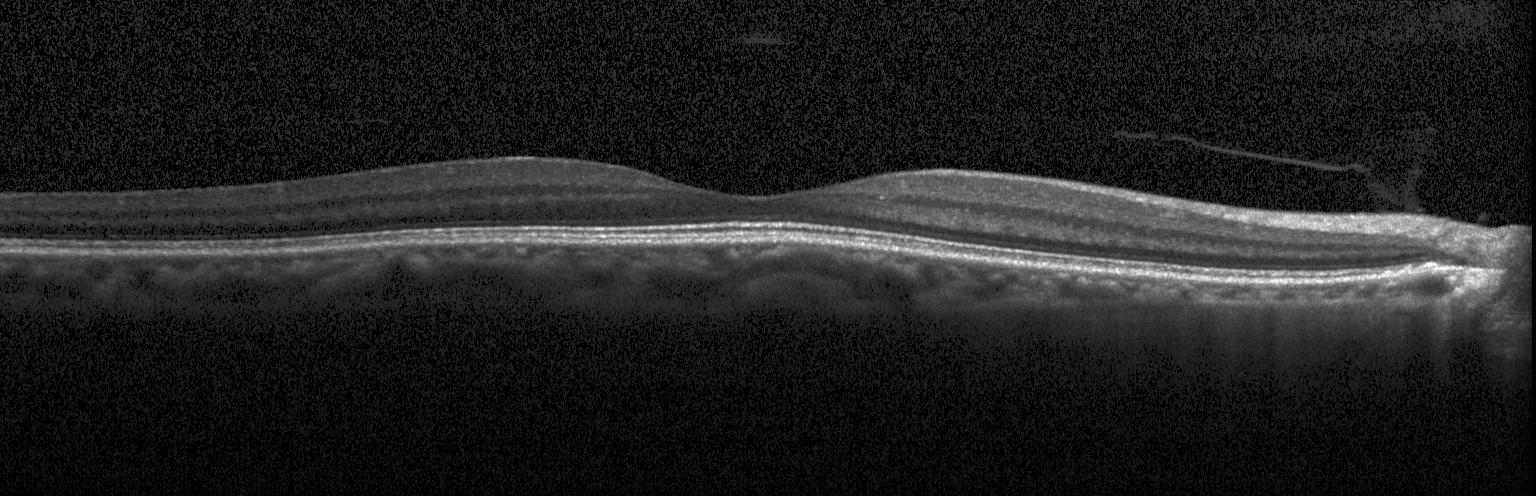
Spectral-domain OCT, retinal OCT B-scan.
Diagnosis: no choroidal neovascularization, no diabetic macular edema, and no drusen.